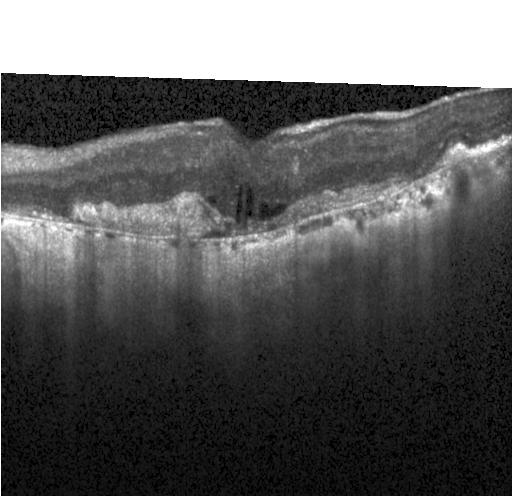 Macular scan; optical coherence tomography B-scan; instrument: Heidelberg Spectralis. Finding: choroidal neovascularization (CNV).